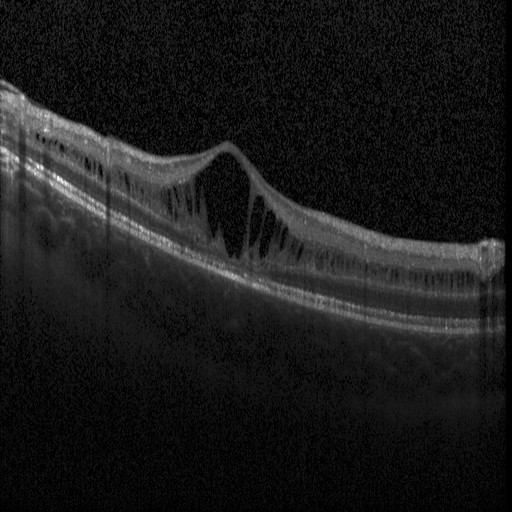 Spectral-domain OCT. Macular scan. Retinal OCT B-scan — Impression: DME.